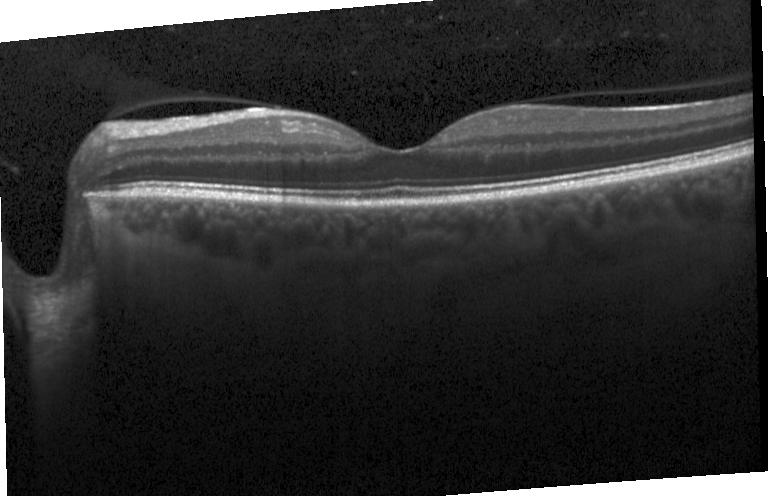 Heidelberg Spectralis OCT system · SD-OCT · optical coherence tomography scan · through the macula.
OCT finding: neither choroidal neovascularization, diabetic macular edema, nor drusen.